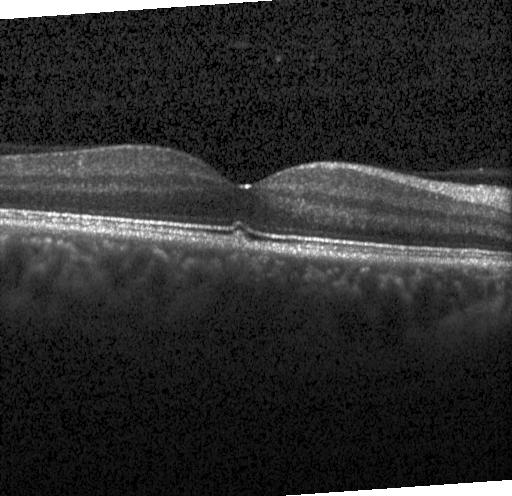
OCT finding: multiple drusen.